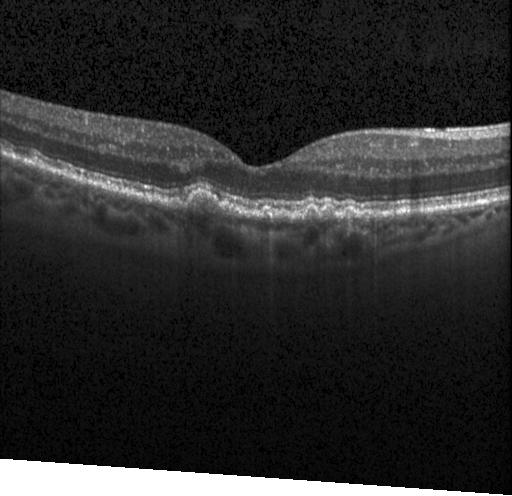
Finding: sub-RPE drusenoid deposits.